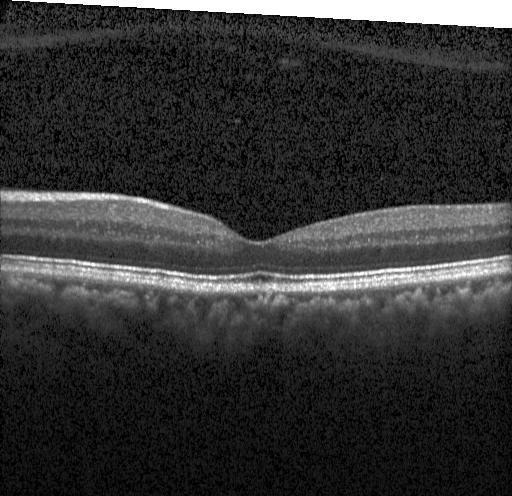 Heidelberg Spectralis. Retinal OCT cross-section. Through the macula. SD-OCT. Finding: no choroidal neovascularization, diabetic macular edema, or drusen.